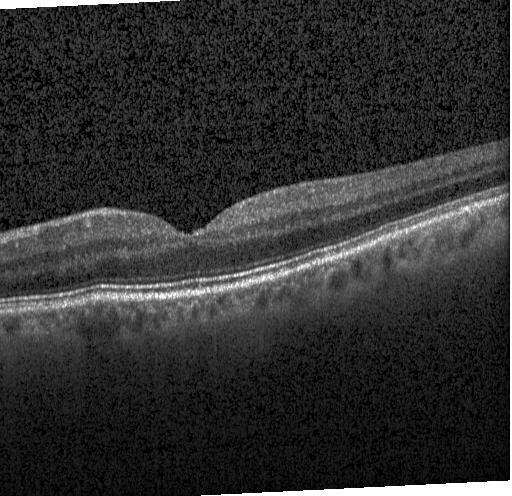

Retinal OCT B-scan, instrument: Heidelberg Spectralis. OCT finding: no choroidal neovascularization, diabetic macular edema, or drusen.